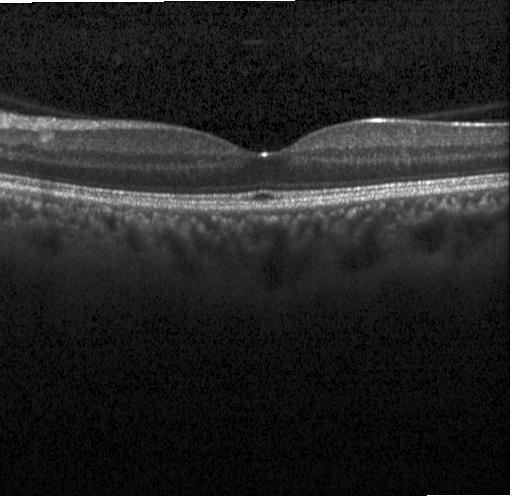

Finding: no evidence of CNV, DME, or drusen.